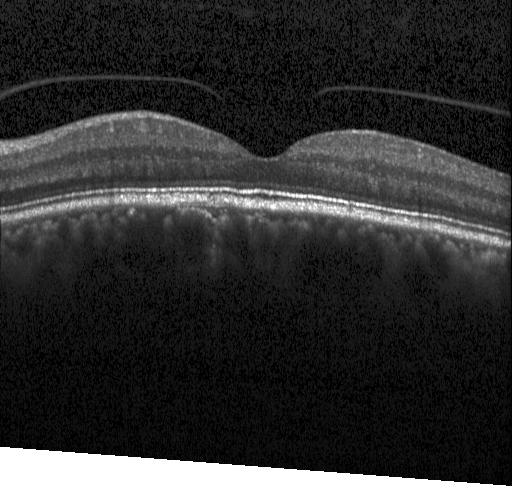
Diagnosis: no choroidal neovascularization, no diabetic macular edema, and no drusen.